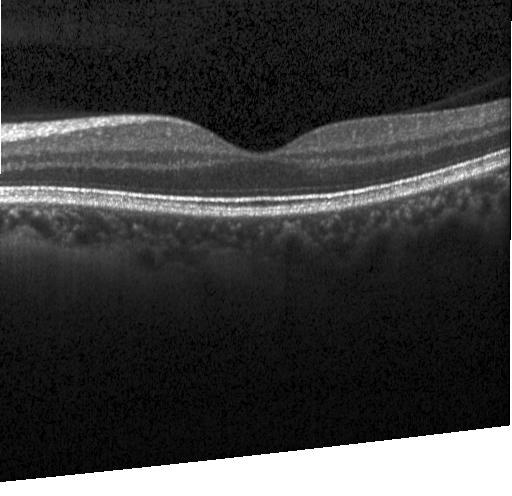 Optical coherence tomography B-scan — The scan shows no evidence of choroidal neovascularization, diabetic macular edema, or drusen.